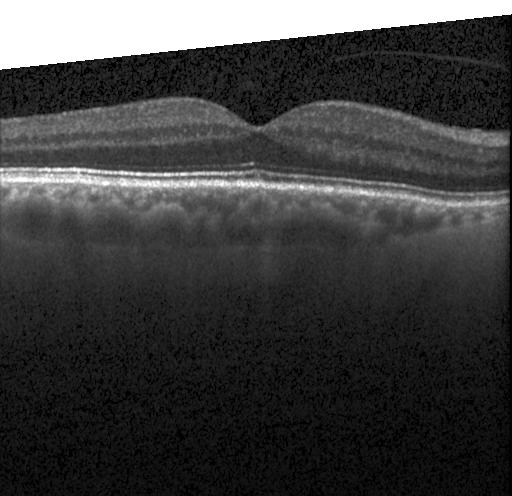

OCT B-scan
OCT finding: neither choroidal neovascularization, diabetic macular edema, nor drusen.